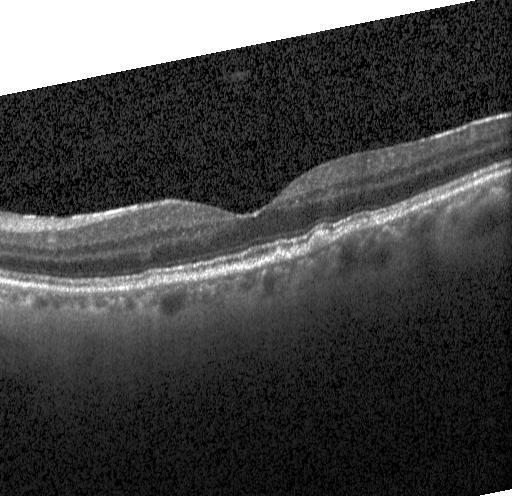
OCT B-scan — The scan shows sub-RPE drusenoid deposits.